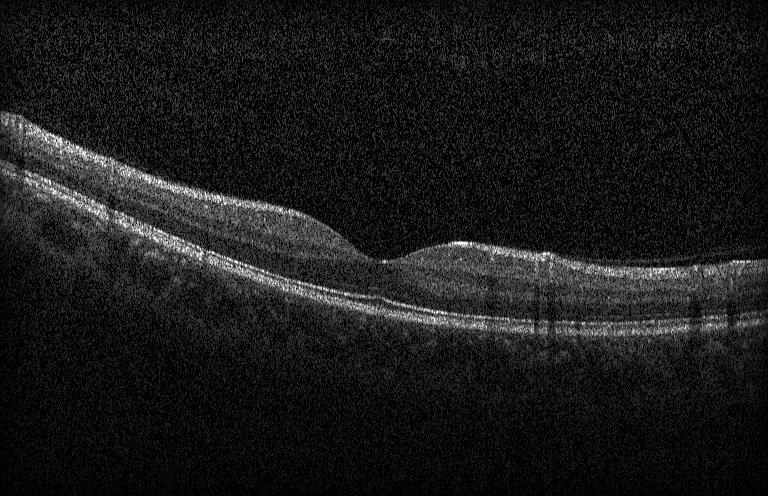
The scan shows no CNV, no DME, and no drusen.